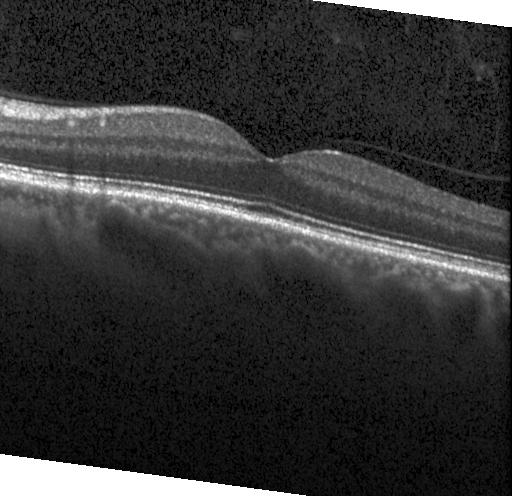

Optical coherence tomography B-scan; instrument: Heidelberg Spectralis; centered on the fovea.
Finding: no CNV, no DME, and no drusen.